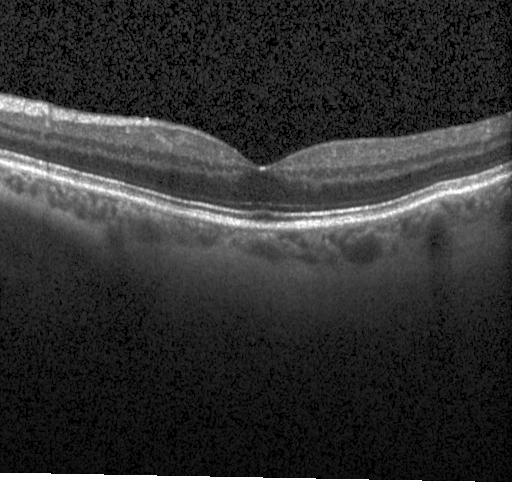
Acquired on a Heidelberg Spectralis · OCT B-scan · fovea-centered · spectral-domain OCT. Finding: no CNV, no DME, and no drusen.